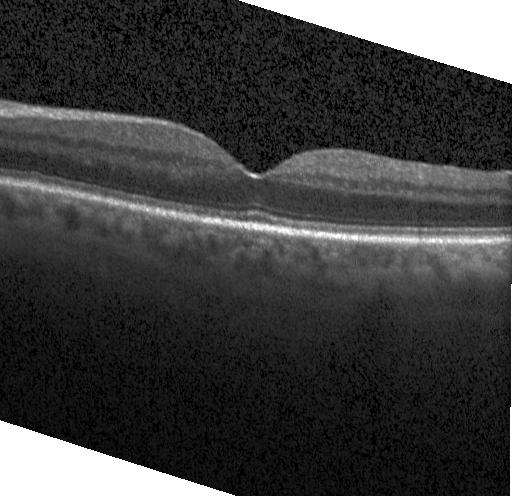
Retinal OCT cross-section. Heidelberg Spectralis OCT system. Spectral-domain OCT. Macular OCT: no choroidal neovascularization, diabetic macular edema, or drusen.